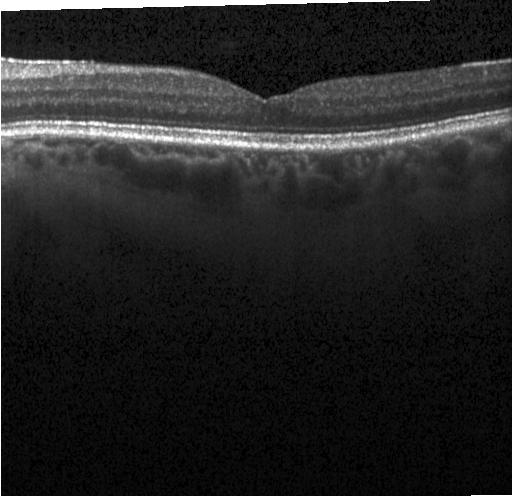 SD-OCT; acquired on a Heidelberg Spectralis; macular scan; optical coherence tomography B-scan — Assessment: no choroidal neovascularization, diabetic macular edema, or drusen.